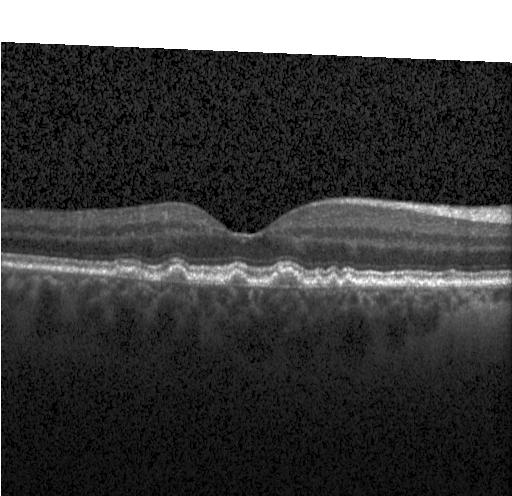

Optical coherence tomography B-scan.
Drusen.